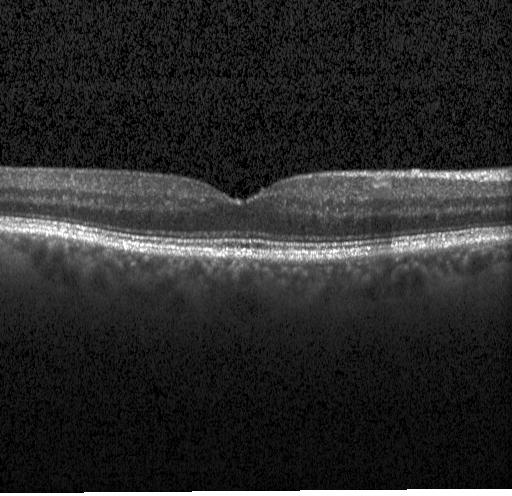 Instrument: Heidelberg Spectralis · retinal OCT cross-section
This B-scan demonstrates no choroidal neovascularization, no diabetic macular edema, and no drusen.